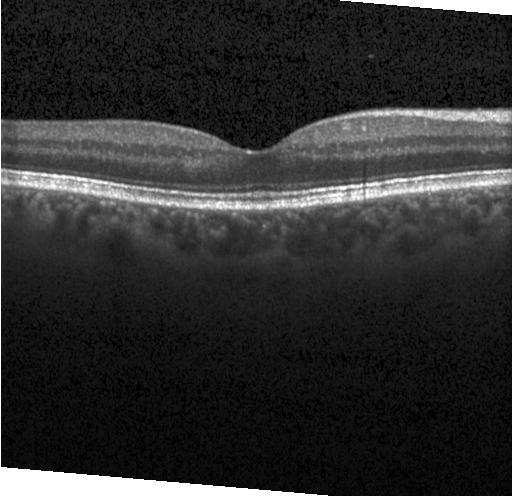

Through the macula. Spectral-domain OCT. Heidelberg Spectralis OCT system. Optical coherence tomography scan.
Diagnosis: no choroidal neovascularization, diabetic macular edema, or drusen.